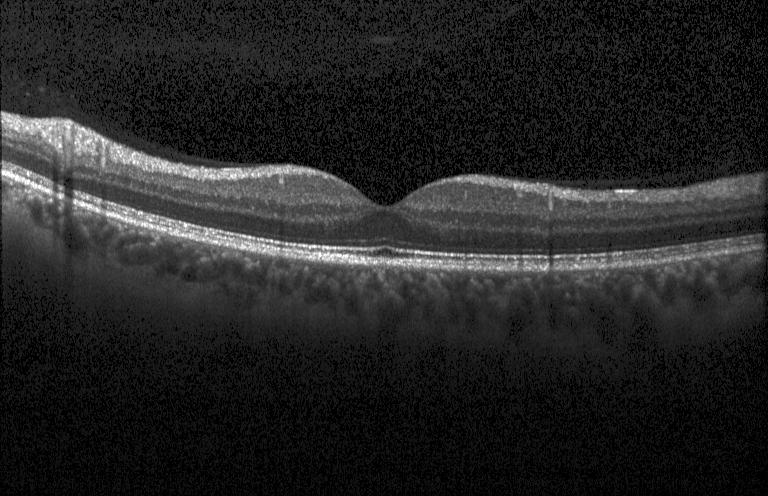
The scan shows no choroidal neovascularization, no diabetic macular edema, and no drusen.